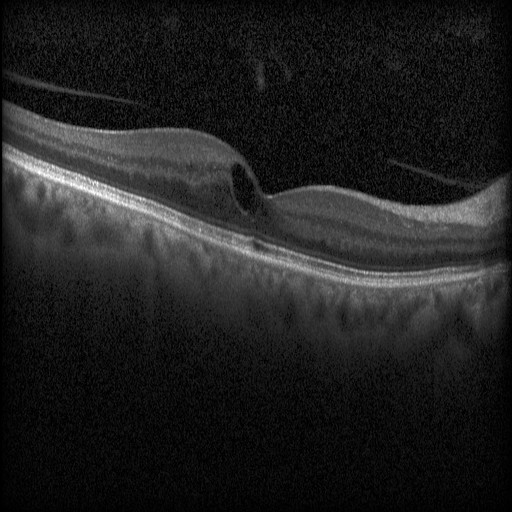
OCT line scan. Heidelberg Spectralis OCT system. Spectral-domain OCT.
DME.